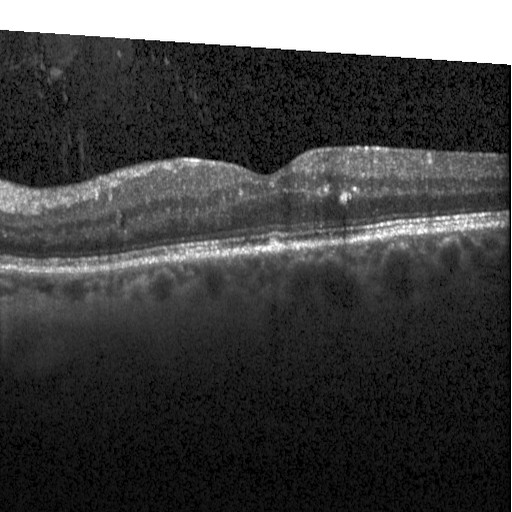 Through the macula. Heidelberg Spectralis. Retinal OCT cross-section
The scan shows DME.